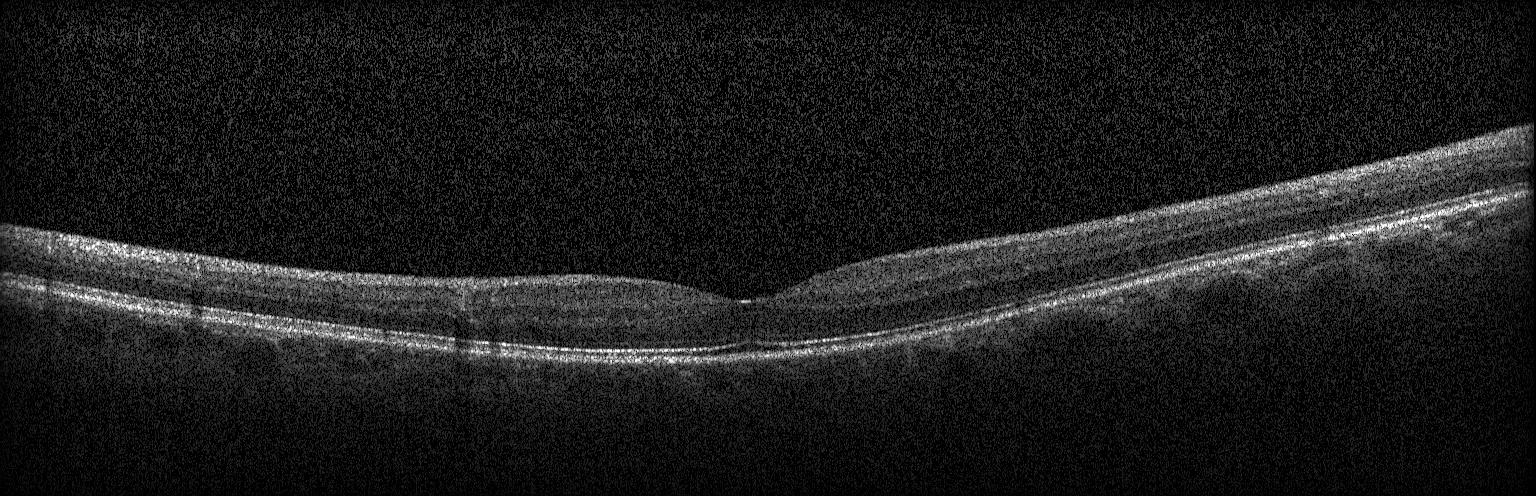

OCT B-scan.
This B-scan demonstrates neither choroidal neovascularization, diabetic macular edema, nor drusen.